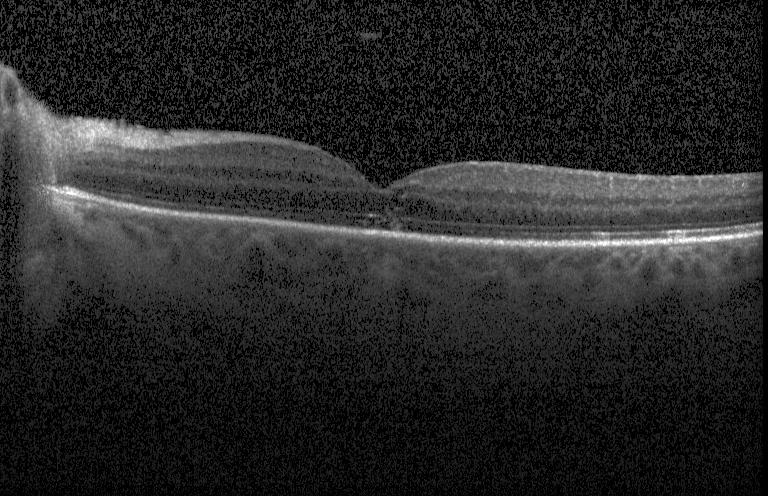
This B-scan demonstrates no evidence of CNV, DME, or drusen.